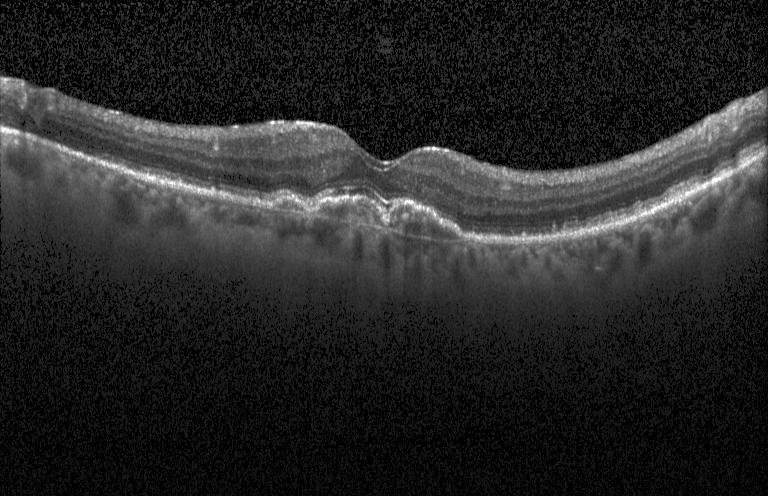 Finding: CNV.